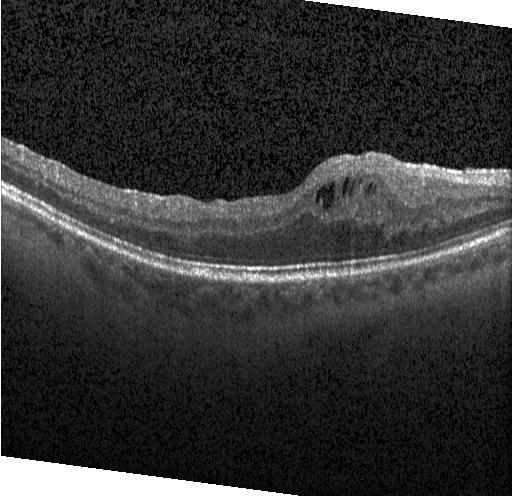

The scan shows DME.